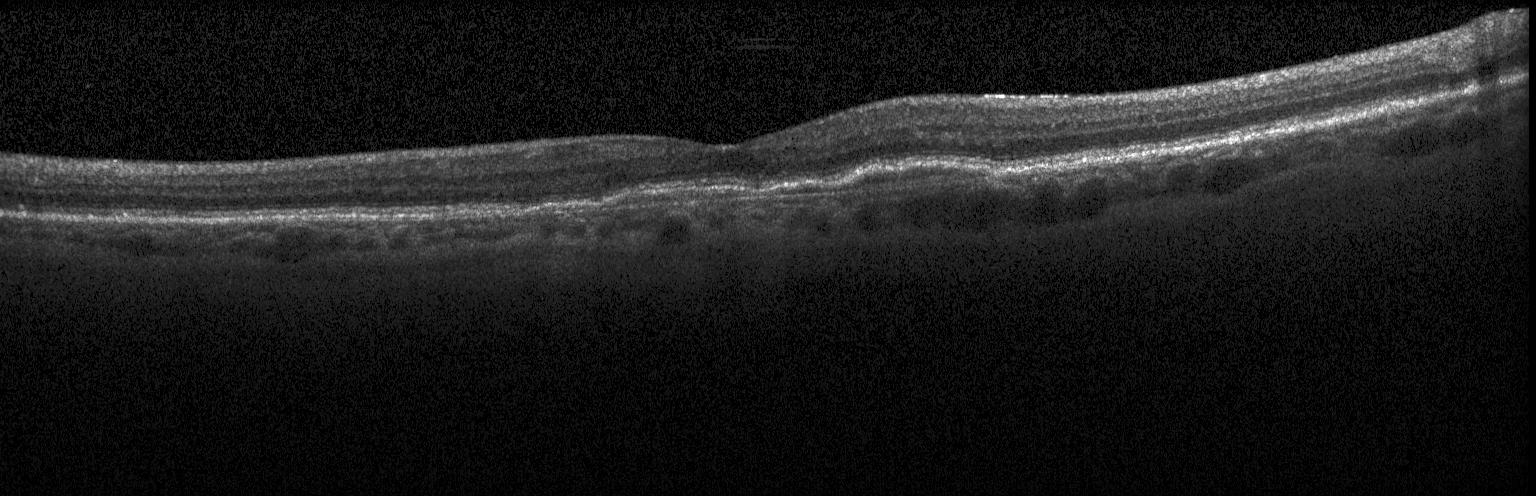 OCT line scan. Heidelberg Spectralis. Spectral-domain OCT. The scan shows a choroidal neovascular membrane.